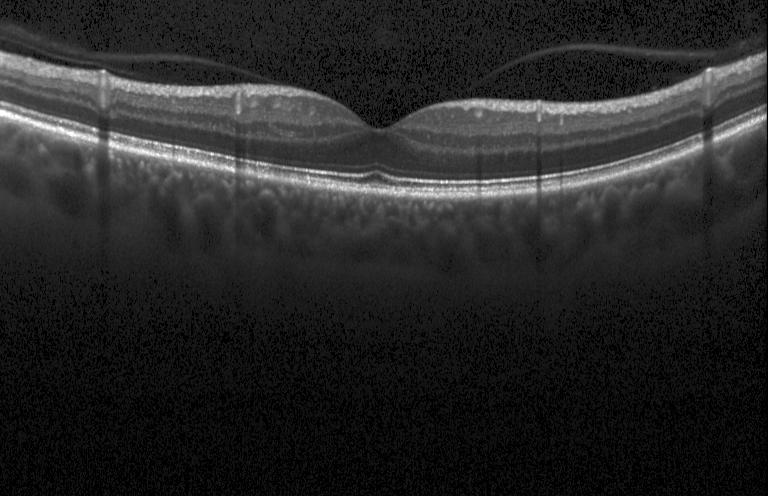

Assessment: no choroidal neovascularization, no diabetic macular edema, and no drusen.